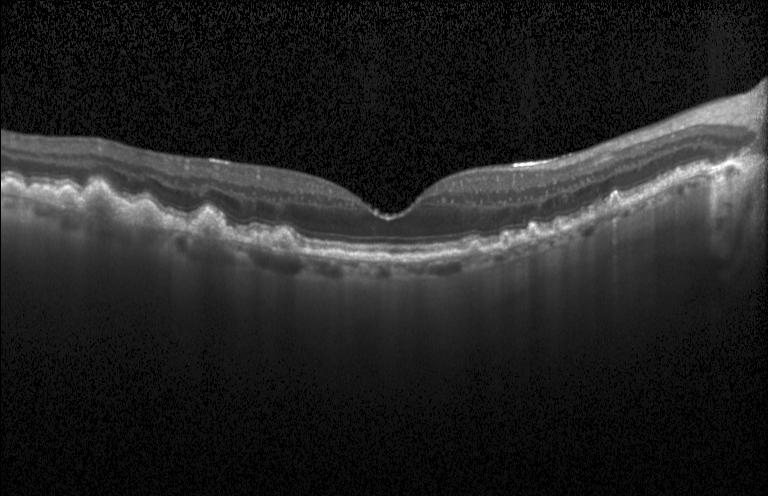

OCT scan showing drusen.